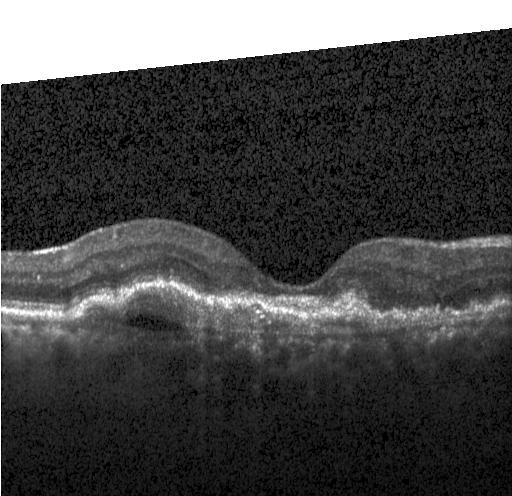
SD-OCT, OCT line scan, through the macula.
Finding: CNV.